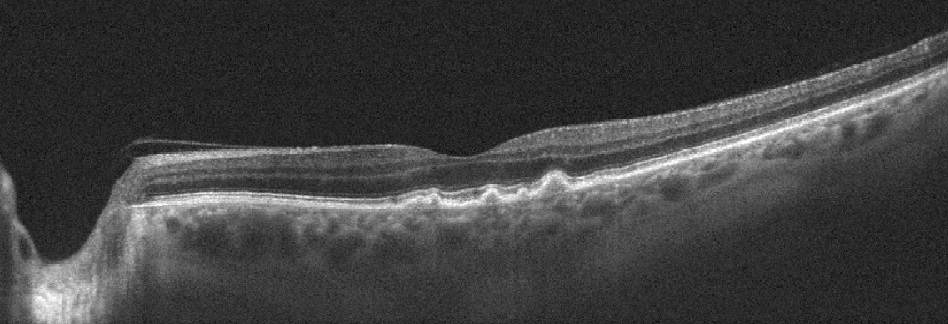

Optovue Avanti RTVue XR · macular scan · optical coherence tomography scan — Macular OCT: age-related macular degeneration.